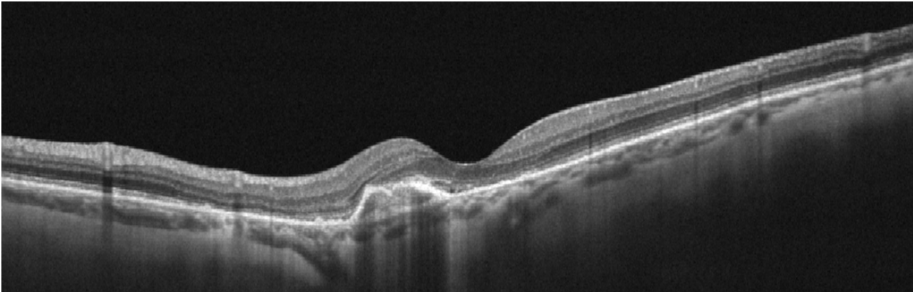 Instrument: Optovue Avanti RTVue XR, optical coherence tomography scan. Macular OCT: age-related macular degeneration.